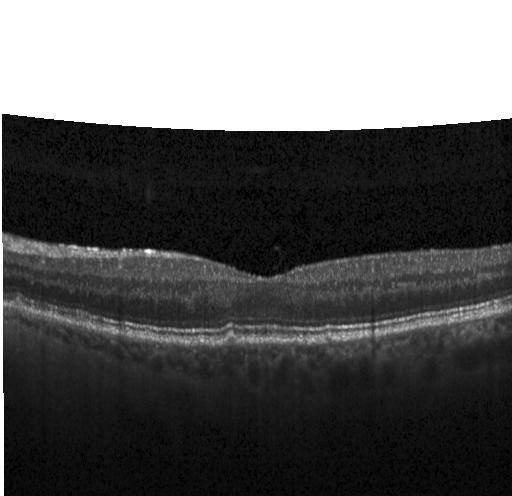

Through the macula · SD-OCT · instrument: Heidelberg Spectralis · OCT B-scan. Finding: drusen.